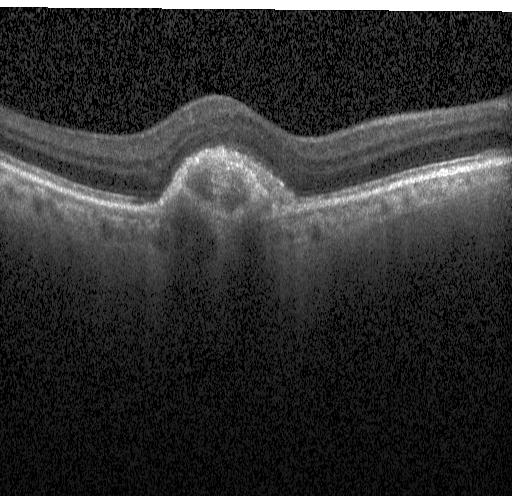
Spectral-domain optical coherence tomography. Retinal OCT B-scan. Macular OCT: a choroidal neovascular membrane.